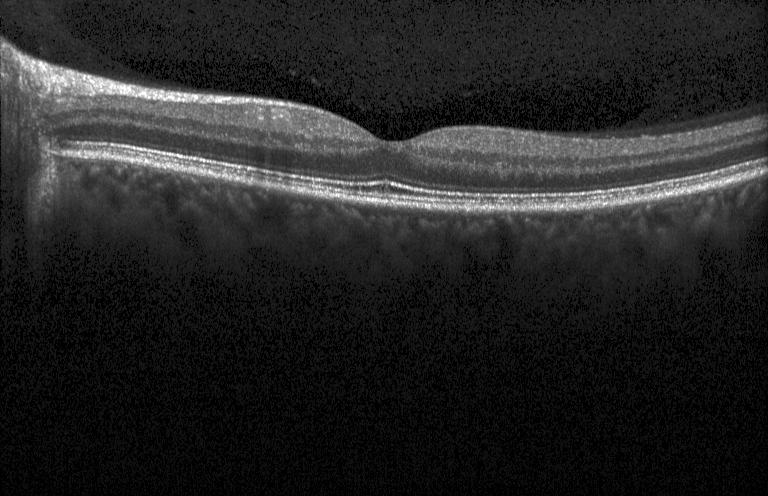 Spectral-domain OCT; horizontal scan through the fovea; optical coherence tomography B-scan
Impression: no CNV, no DME, and no drusen.